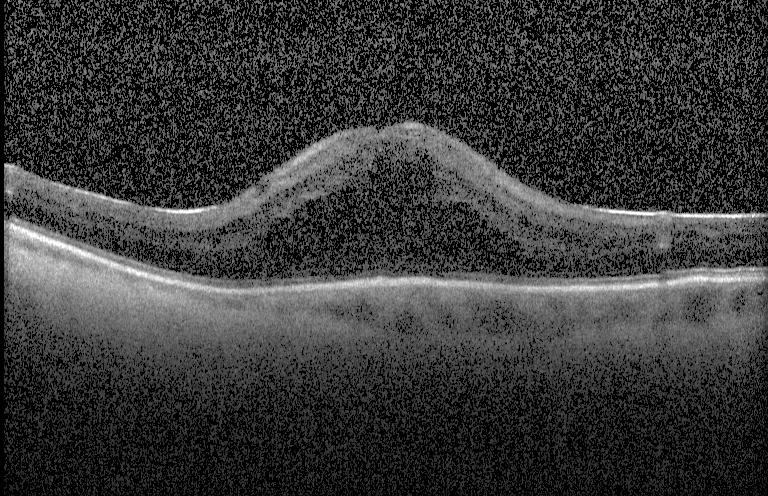
Finding: DME.